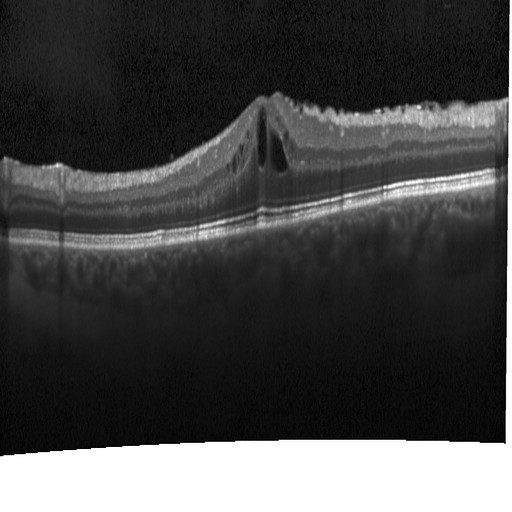

Diagnosis: DME.